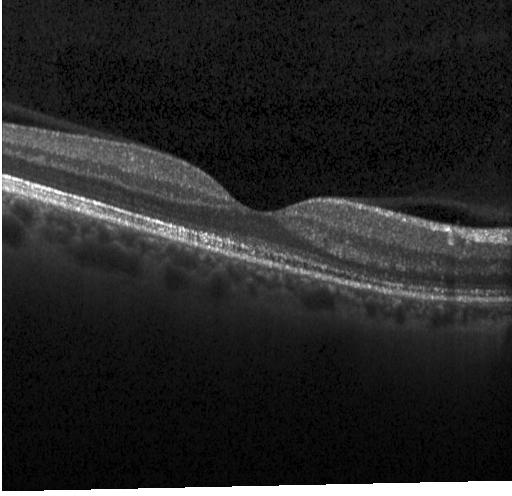
Through the macula · SD-OCT · optical coherence tomography scan · acquired on a Heidelberg Spectralis
This B-scan demonstrates neither choroidal neovascularization, diabetic macular edema, nor drusen.